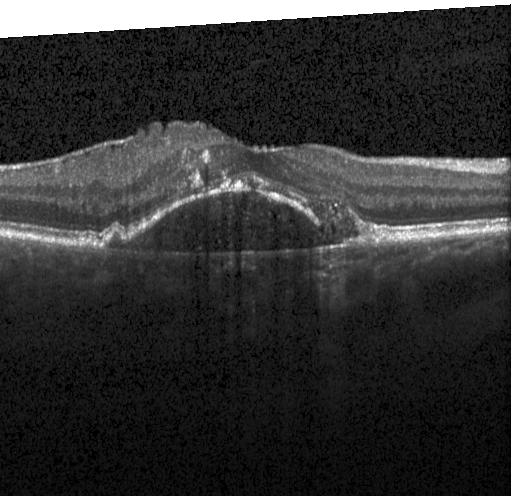

Impression: CNV.